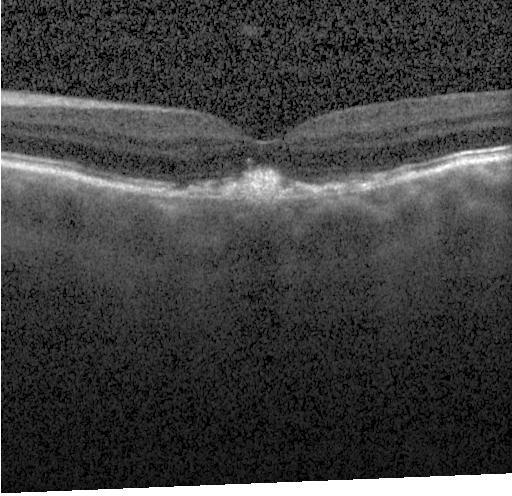
Assessment: choroidal neovascularization.